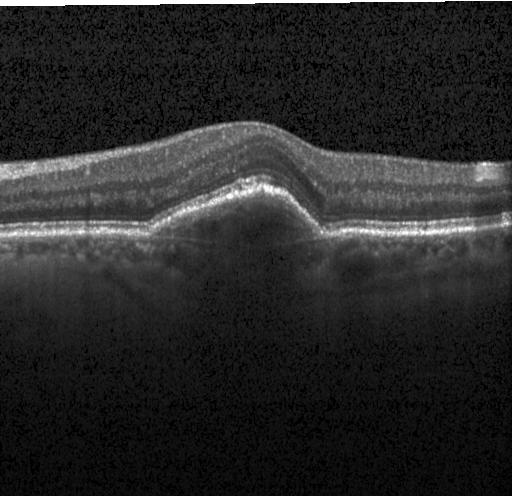

Optical coherence tomography B-scan.
Finding: a choroidal neovascular membrane.